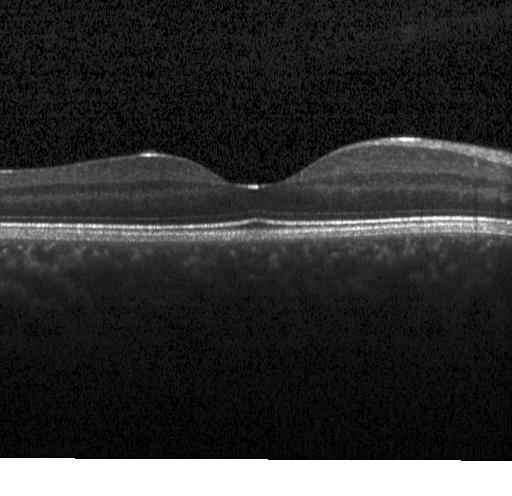
Optical coherence tomography B-scan. Assessment: no evidence of choroidal neovascularization, diabetic macular edema, or drusen.